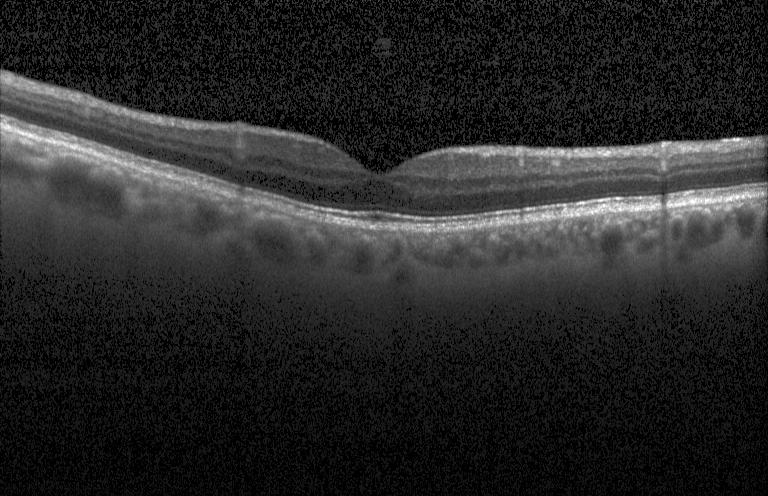

Optical coherence tomography B-scan · Heidelberg Spectralis OCT system · spectral-domain optical coherence tomography · through the macula
Dx: no choroidal neovascularization, no diabetic macular edema, and no drusen.